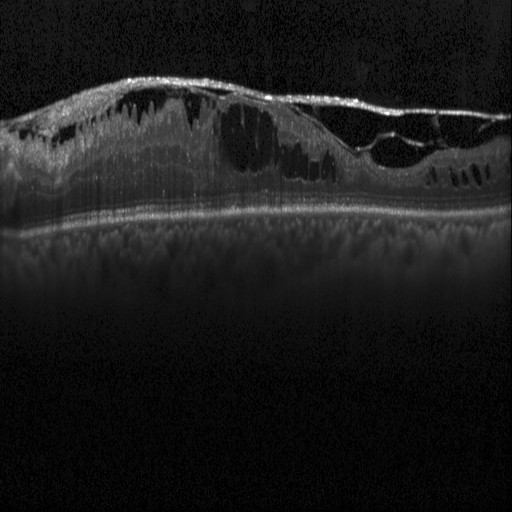
Fovea-centered. OCT B-scan
Dx: diabetic macular edema (DME).